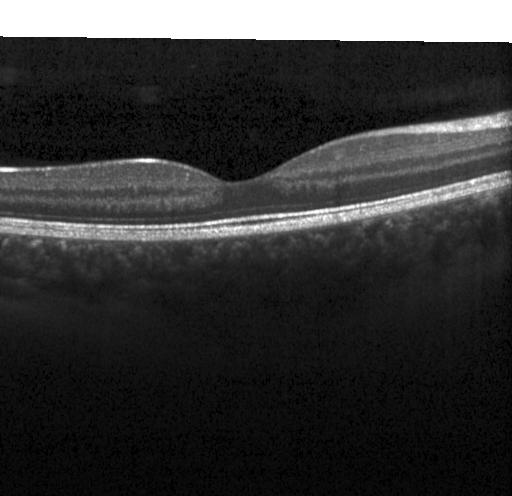

Impression: no evidence of CNV, DME, or drusen.